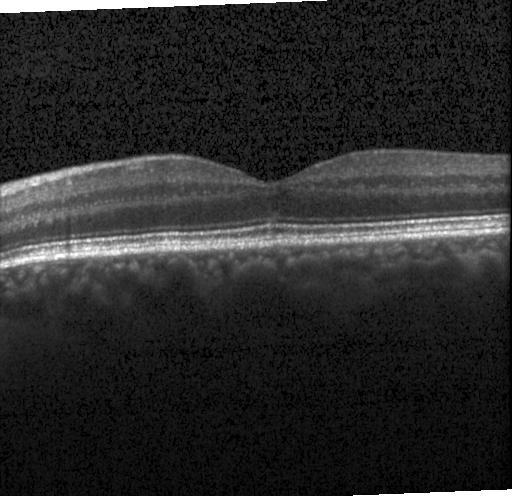 Heidelberg Spectralis · retinal OCT cross-section · centered on the fovea · spectral-domain OCT — Finding: neither choroidal neovascularization, diabetic macular edema, nor drusen.